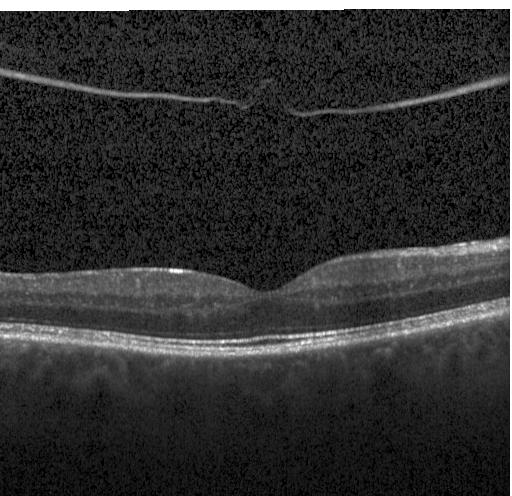 OCT scan showing no CNV, DME, or drusen.